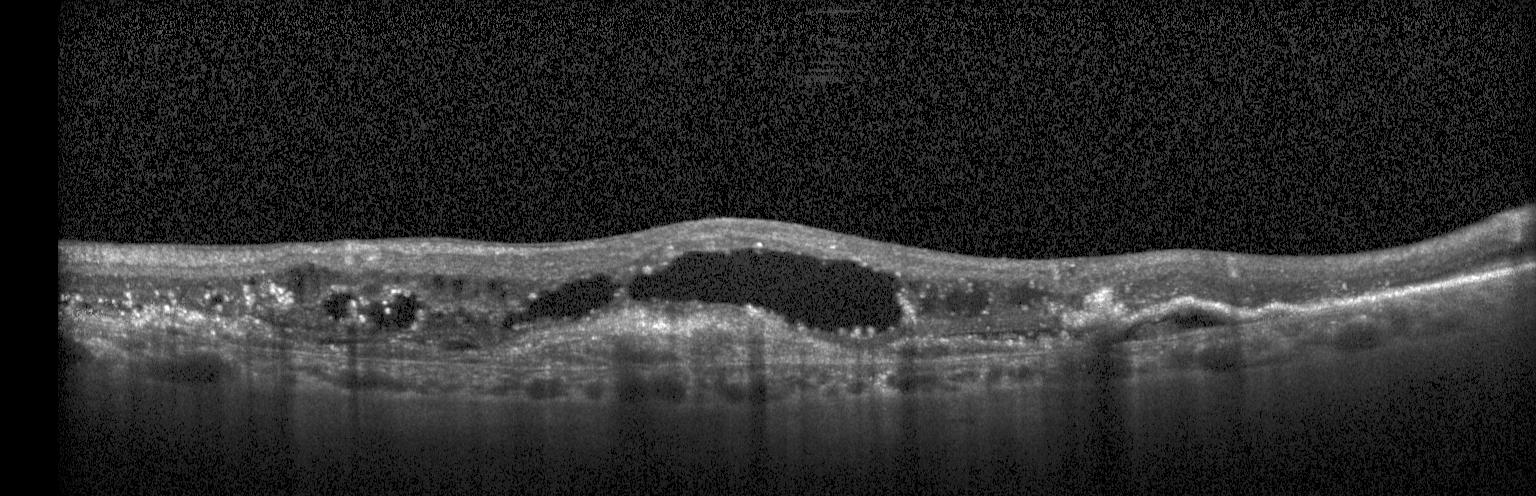
Heidelberg Spectralis OCT system, optical coherence tomography scan — Assessment: choroidal neovascularization.